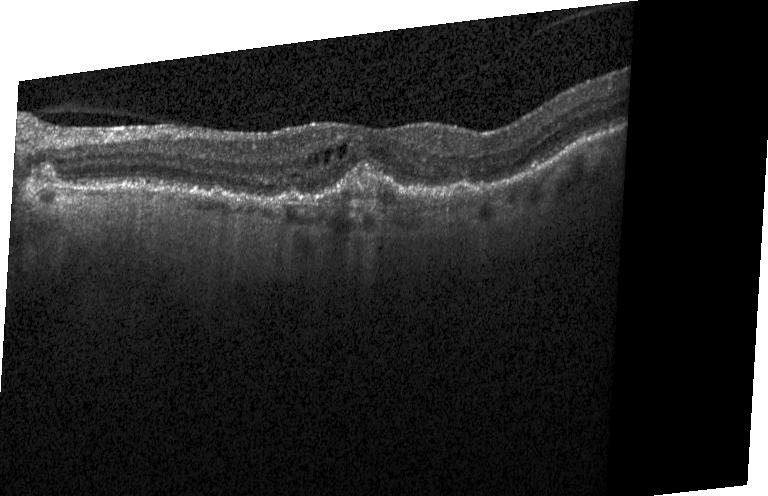 Through the macula. Instrument: Heidelberg Spectralis. SD-OCT. OCT B-scan
Diagnosis: a choroidal neovascular membrane.